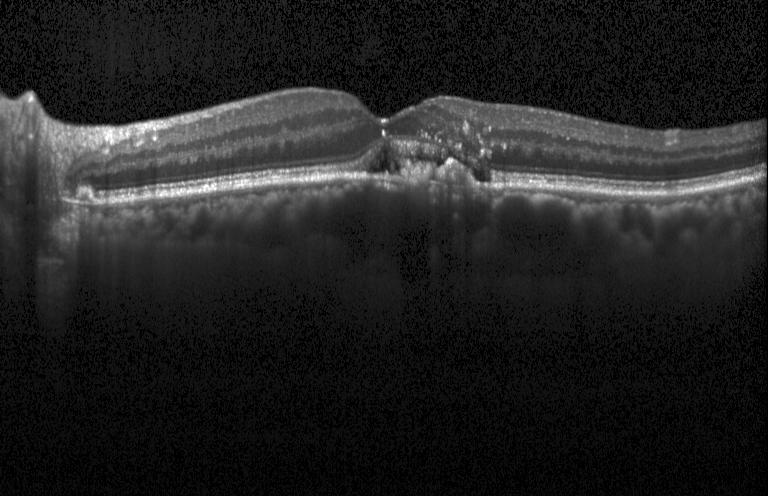

Instrument: Heidelberg Spectralis · centered on the fovea · spectral-domain OCT · optical coherence tomography scan
The scan shows a choroidal neovascular membrane.